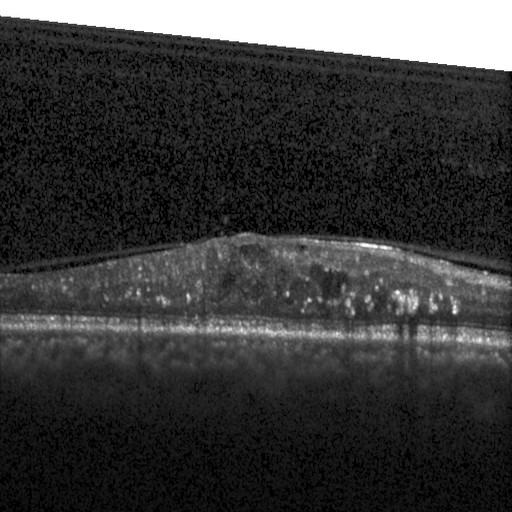
Fovea-centered · retinal OCT B-scan. Diabetic macular edema.